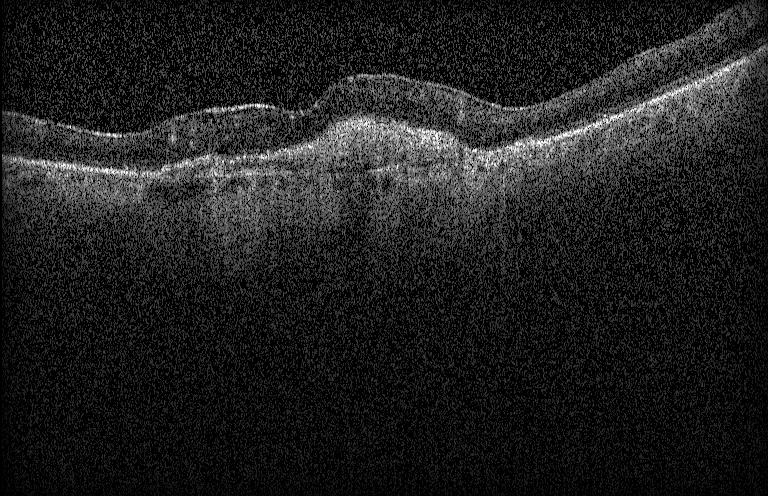

Retinal OCT cross-section showing a choroidal neovascular membrane.